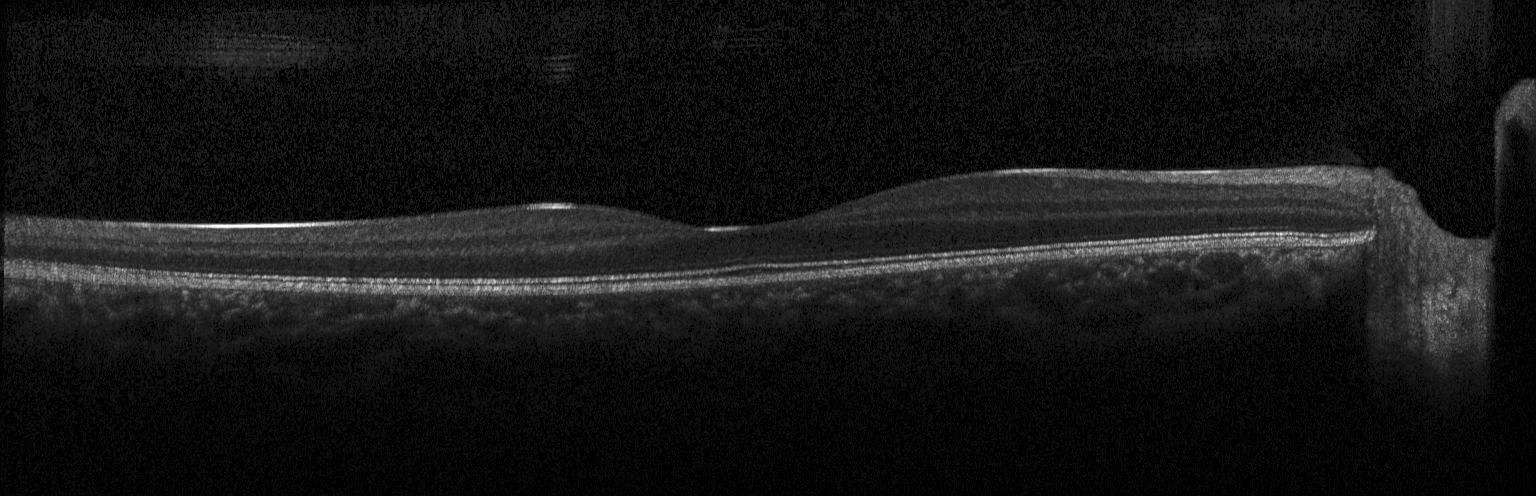
Macular scan, OCT line scan, spectral-domain optical coherence tomography. Diagnosis: no CNV, DME, or drusen.